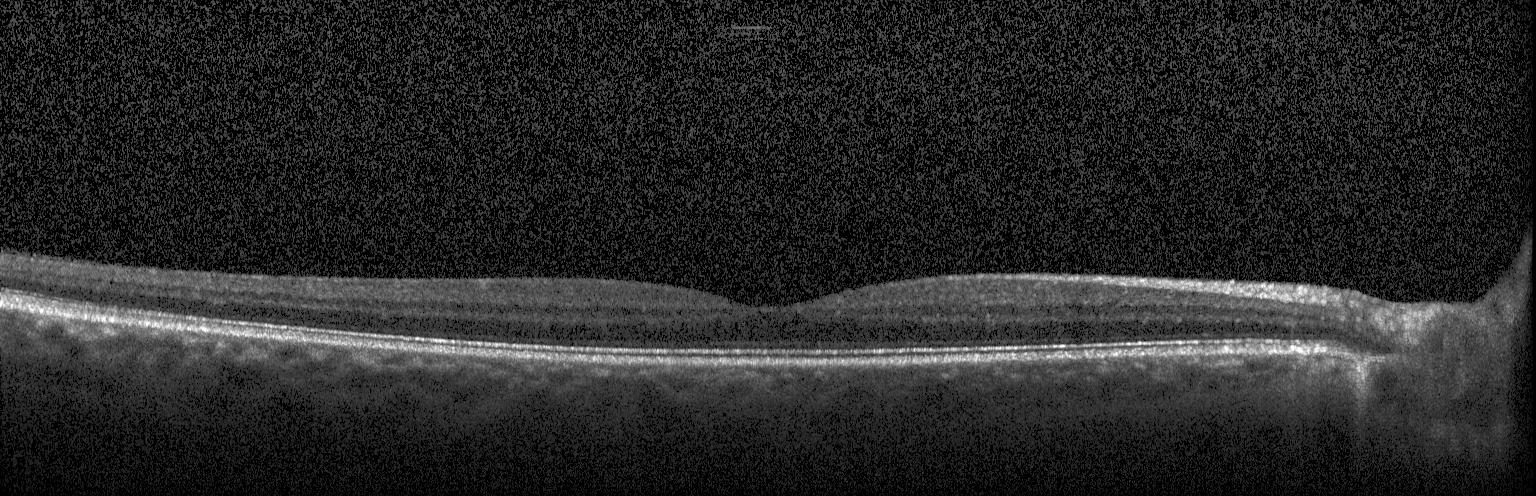
OCT scan showing no CNV, no DME, and no drusen.